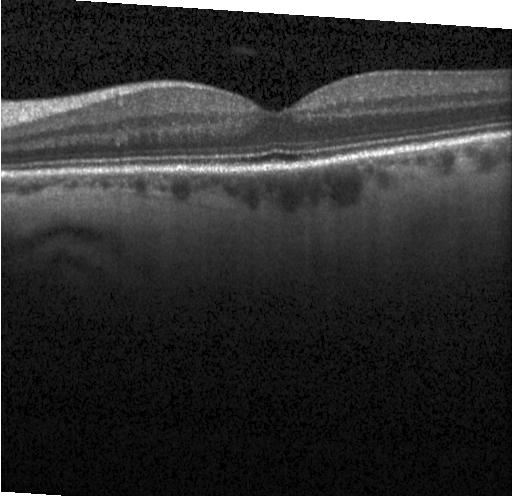
No choroidal neovascularization, diabetic macular edema, or drusen.